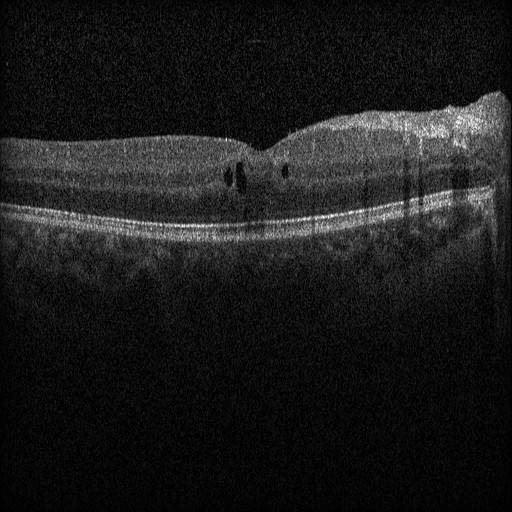

This B-scan demonstrates DME.